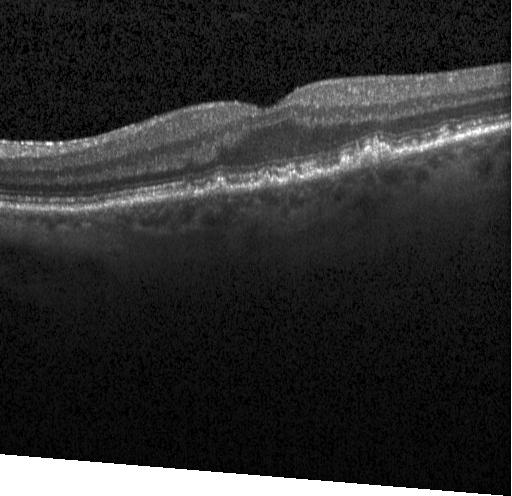

Retinal OCT B-scan. Through the macula — This B-scan demonstrates sub-RPE drusenoid deposits.